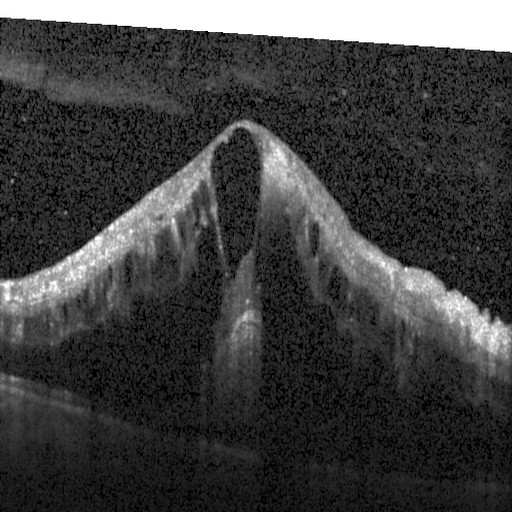

Macular OCT: diabetic macular edema.